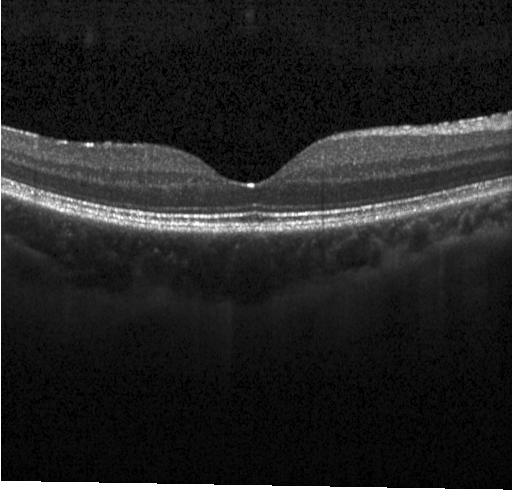
OCT B-scan showing no evidence of CNV, DME, or drusen.